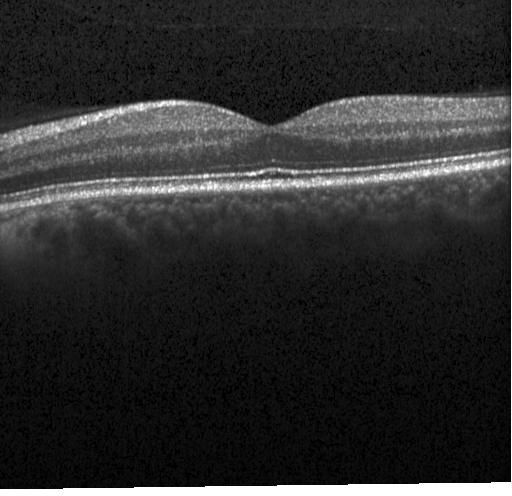 This B-scan demonstrates no choroidal neovascularization, diabetic macular edema, or drusen.